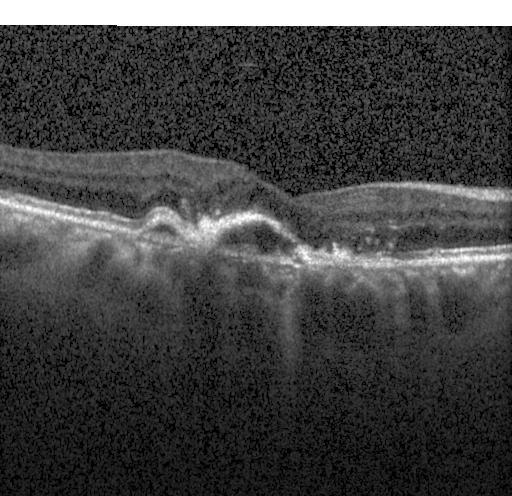 Fovea-centered, retinal OCT B-scan
Dx: choroidal neovascularization (CNV).